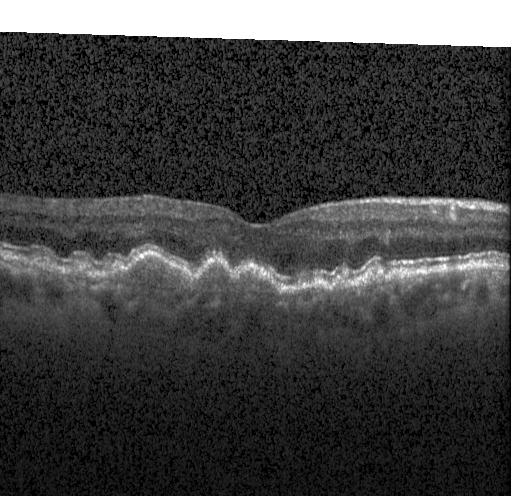

Retinal OCT cross-section showing sub-RPE drusenoid deposits.